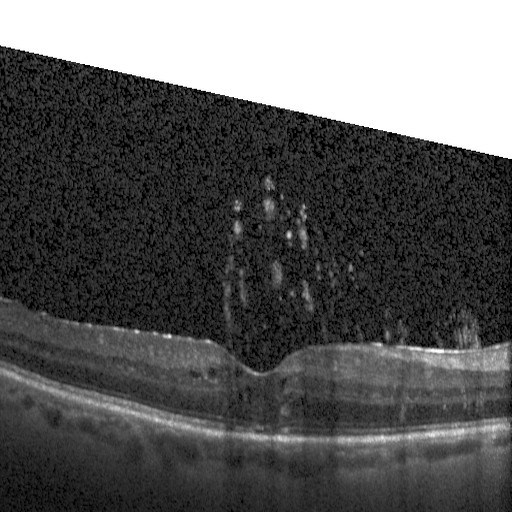

OCT B-scan showing diabetic macular edema (DME).